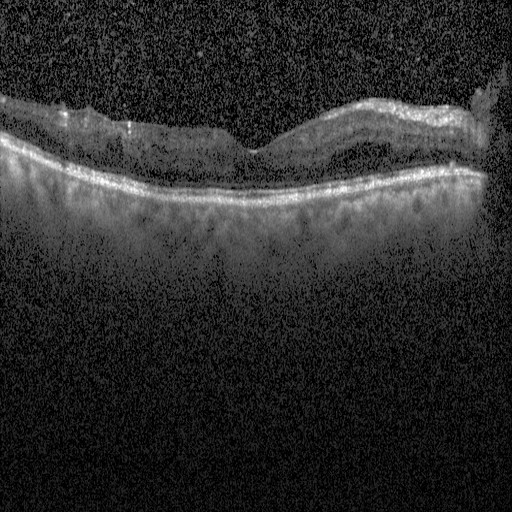 Centered on the fovea; Heidelberg Spectralis OCT system; spectral-domain optical coherence tomography; optical coherence tomography scan.
Assessment: diabetic macular edema (DME).